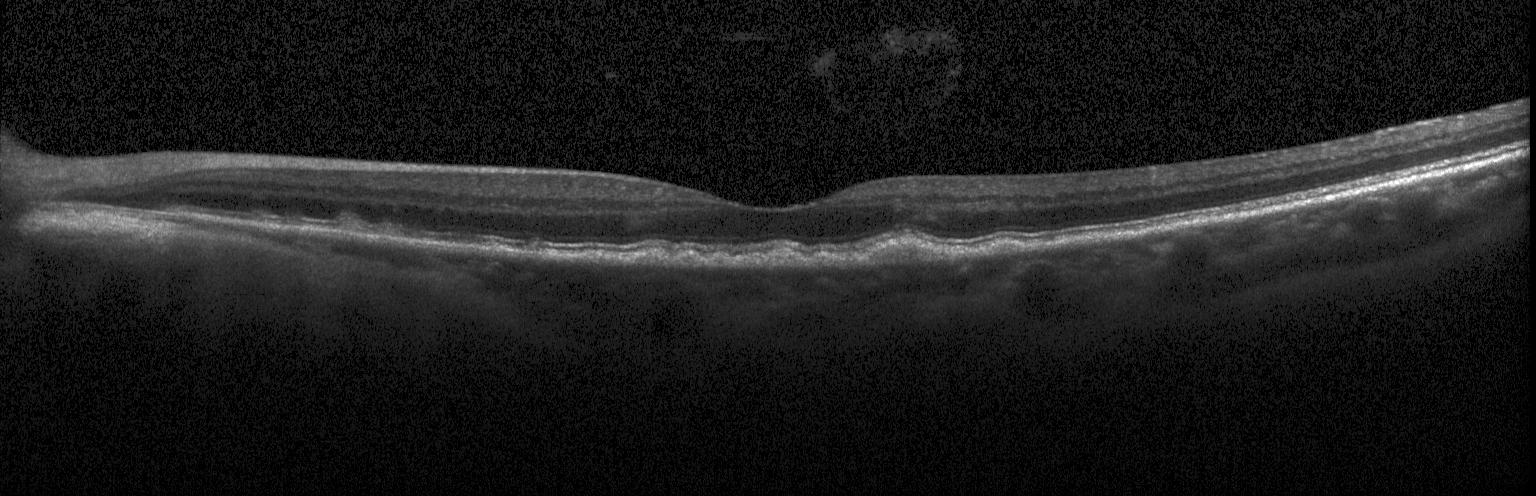

Macular scan; instrument: Heidelberg Spectralis; spectral-domain optical coherence tomography; retinal OCT cross-section. Assessment: drusen.